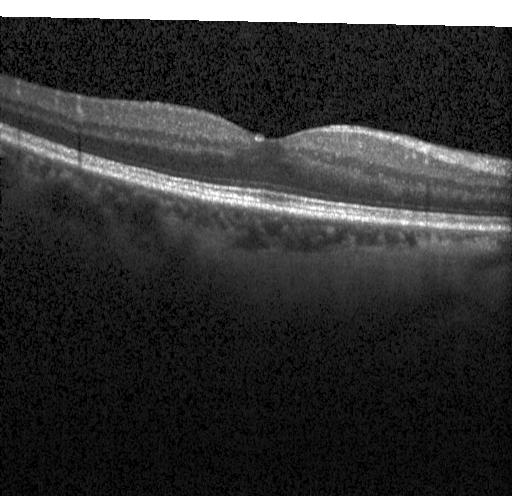

OCT line scan. Finding: no evidence of choroidal neovascularization, diabetic macular edema, or drusen.